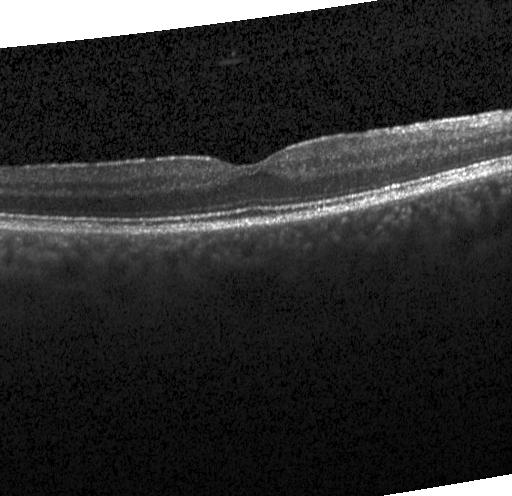

Assessment: no evidence of choroidal neovascularization, diabetic macular edema, or drusen.